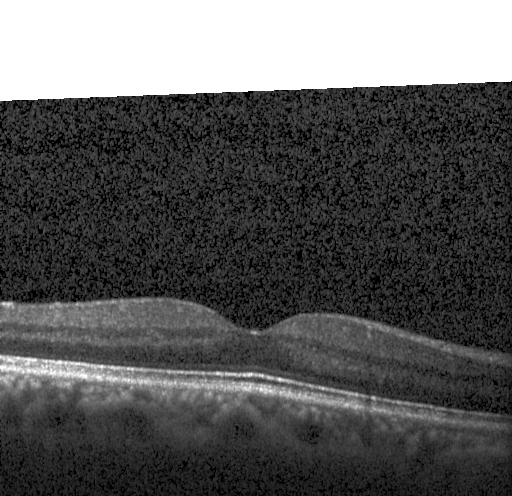 Spectral-domain OCT B-scan: no CNV, no DME, and no drusen.